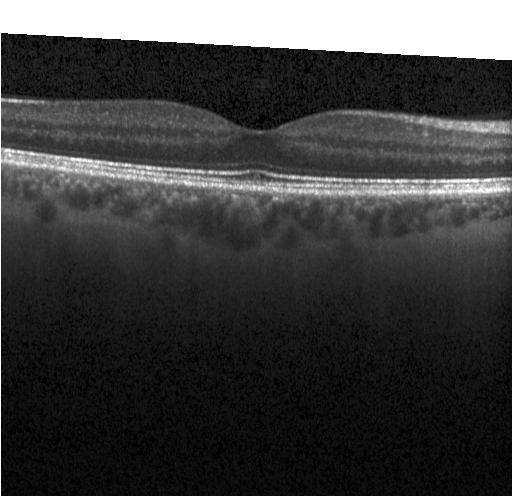
Retinal OCT B-scan, spectral-domain optical coherence tomography, through the macula
No CNV, DME, or drusen.